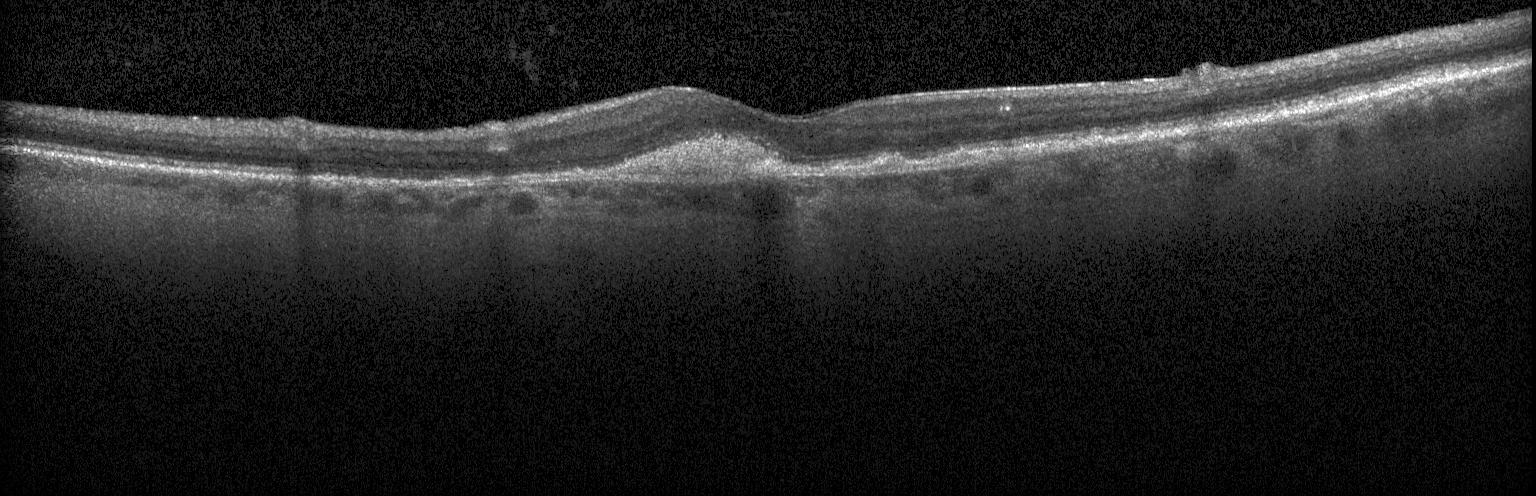
Macular OCT demonstrating choroidal neovascularization.